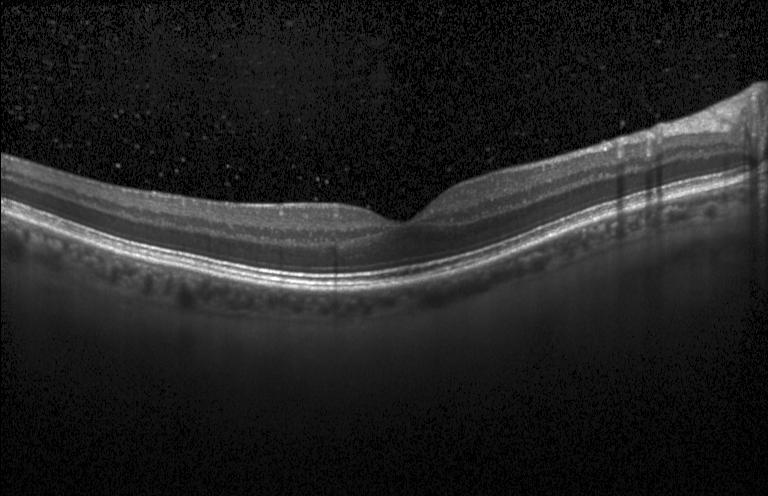
Macular OCT demonstrating neither CNV, DME, nor drusen.